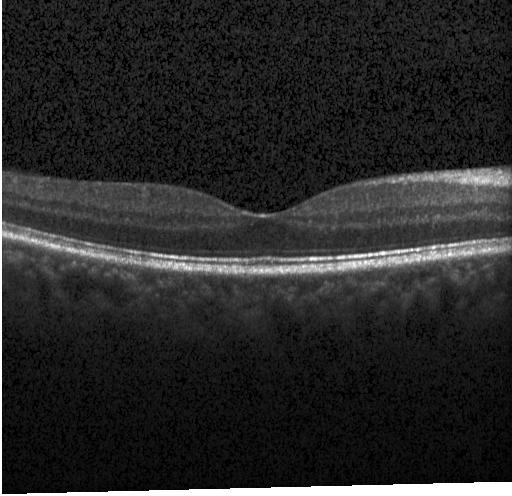 Fovea-centered, OCT line scan — Diagnosis: no evidence of CNV, DME, or drusen.